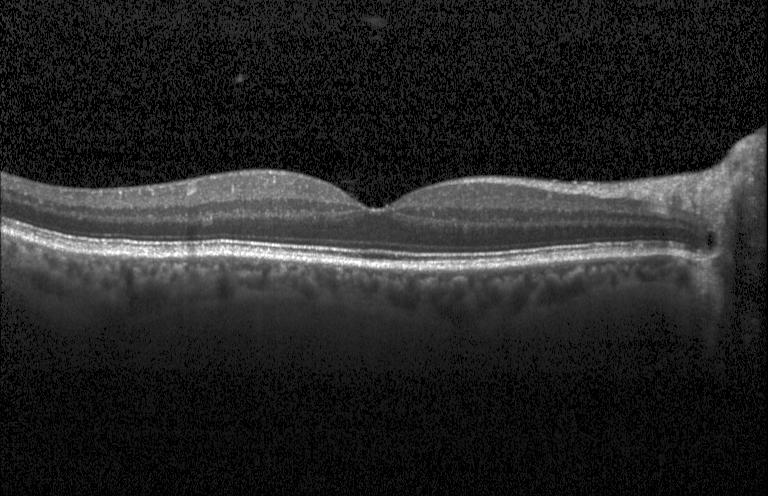
Finding: no evidence of CNV, DME, or drusen.